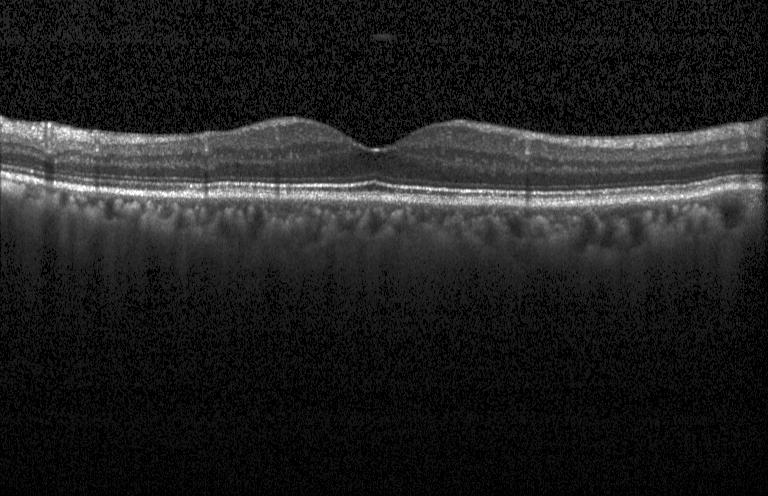 Optical coherence tomography scan · spectral-domain optical coherence tomography — Diagnosis: neither choroidal neovascularization, diabetic macular edema, nor drusen.